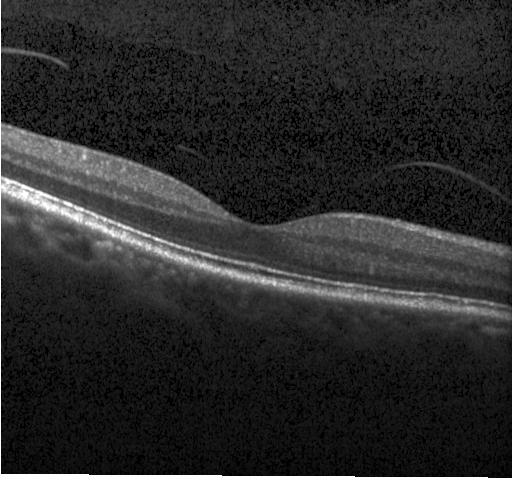 Finding: neither choroidal neovascularization, diabetic macular edema, nor drusen.